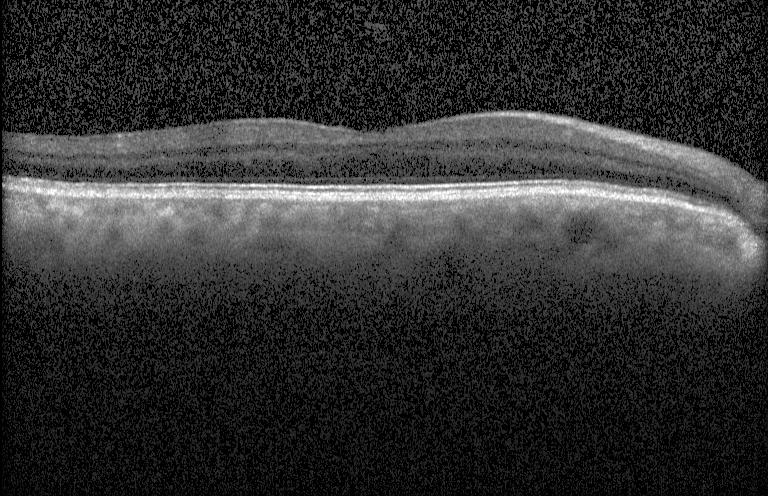 Diagnosis: no choroidal neovascularization, no diabetic macular edema, and no drusen.